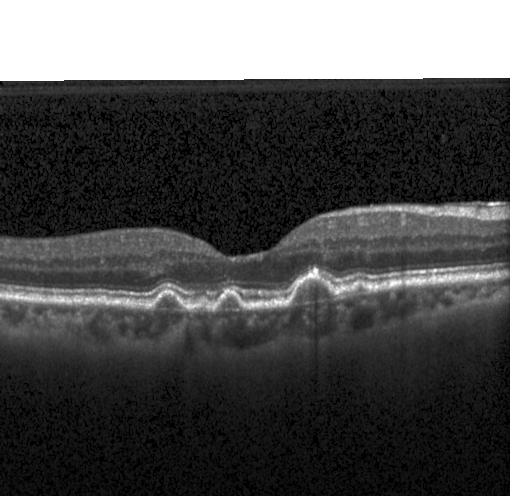

OCT B-scan showing multiple drusen.